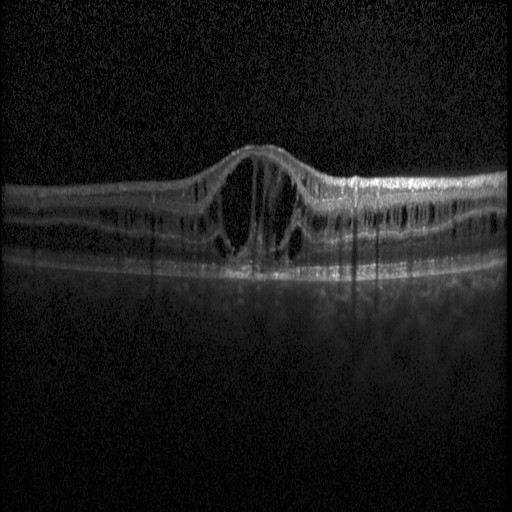

Retinal OCT cross-section, acquired on a Heidelberg Spectralis, spectral-domain optical coherence tomography
This B-scan demonstrates diabetic macular edema.